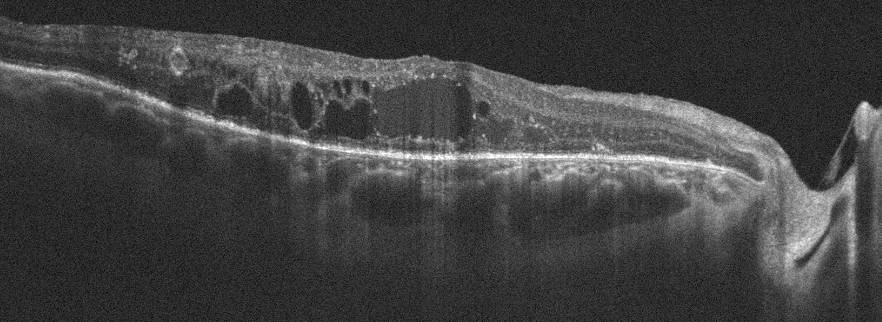
Through the macula, retinal OCT B-scan, oculus dexter, acquired on an Optovue Avanti RTVue XR. The scan shows diabetic macular edema.